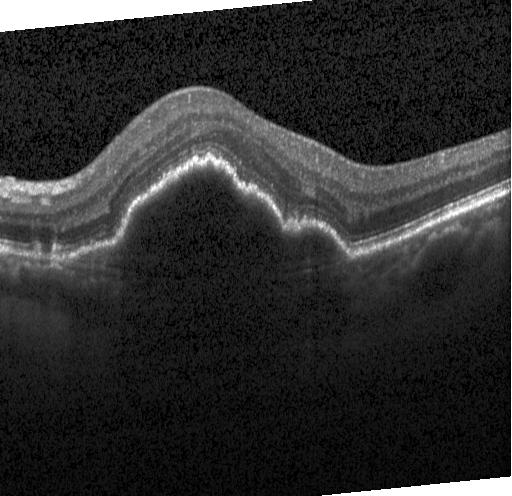
Choroidal neovascularization.